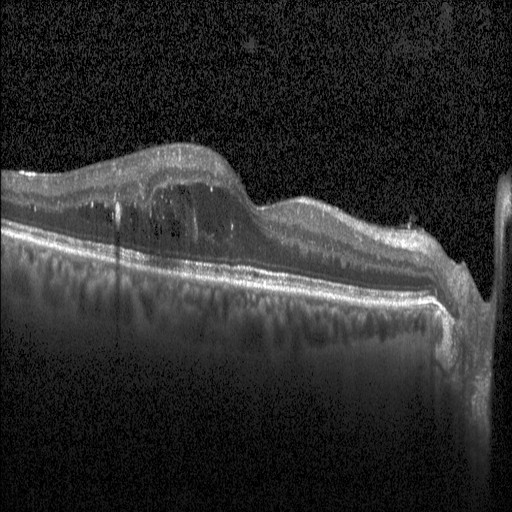 Spectral-domain OCT. Retinal OCT cross-section — Dx: DME.